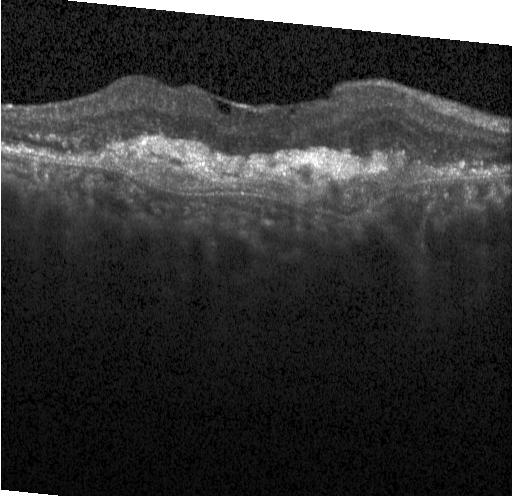

Acquired on a Heidelberg Spectralis. Optical coherence tomography B-scan. Horizontal scan through the fovea. Spectral-domain OCT. Finding: choroidal neovascularization.